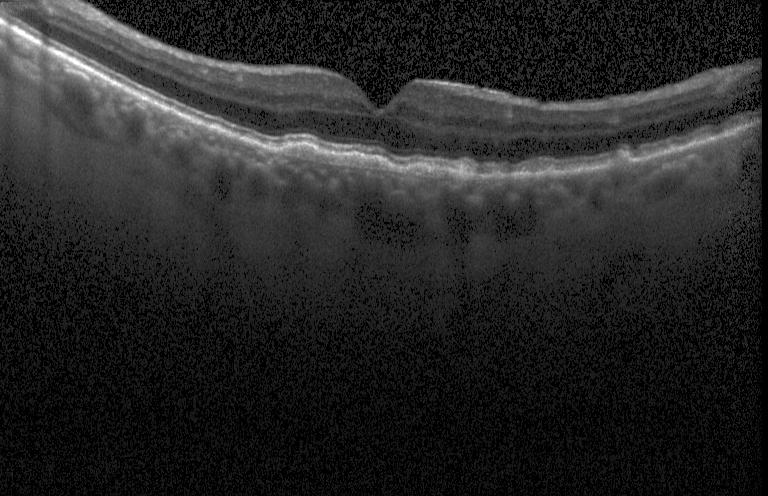 Finding: a choroidal neovascular membrane.